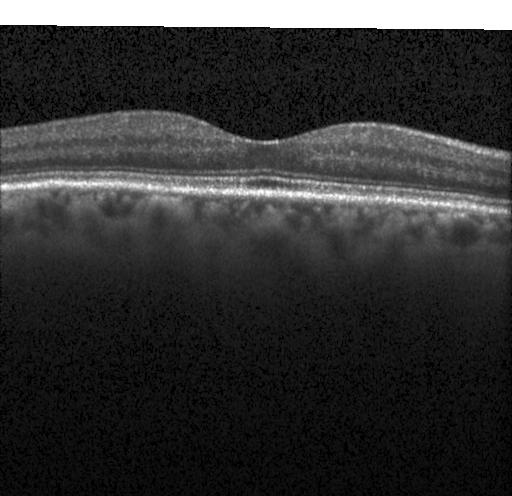 Fovea-centered; instrument: Heidelberg Spectralis; optical coherence tomography scan. Impression: no CNV, DME, or drusen.